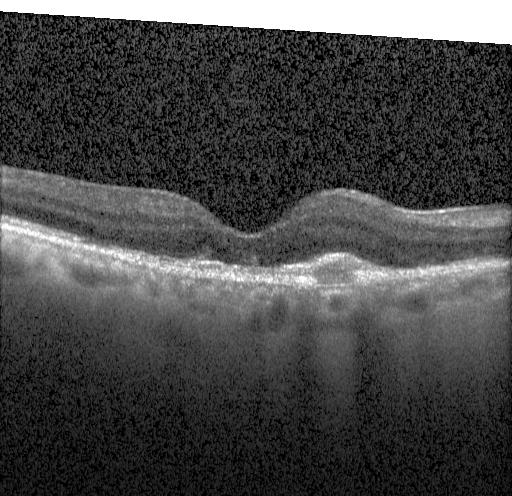 Retinal OCT cross-section showing a choroidal neovascular membrane.